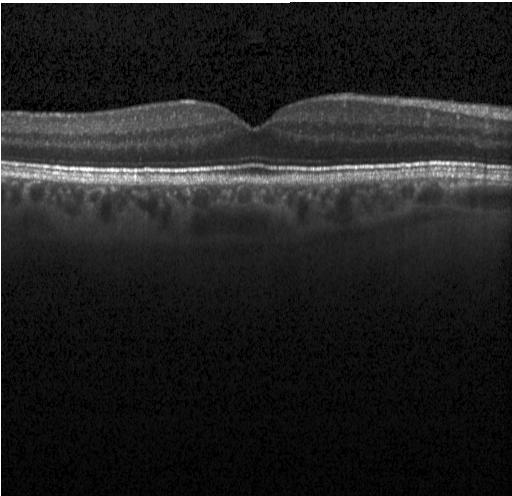 Acquired on a Heidelberg Spectralis; macular scan; spectral-domain OCT; optical coherence tomography scan
This B-scan demonstrates no evidence of choroidal neovascularization, diabetic macular edema, or drusen.